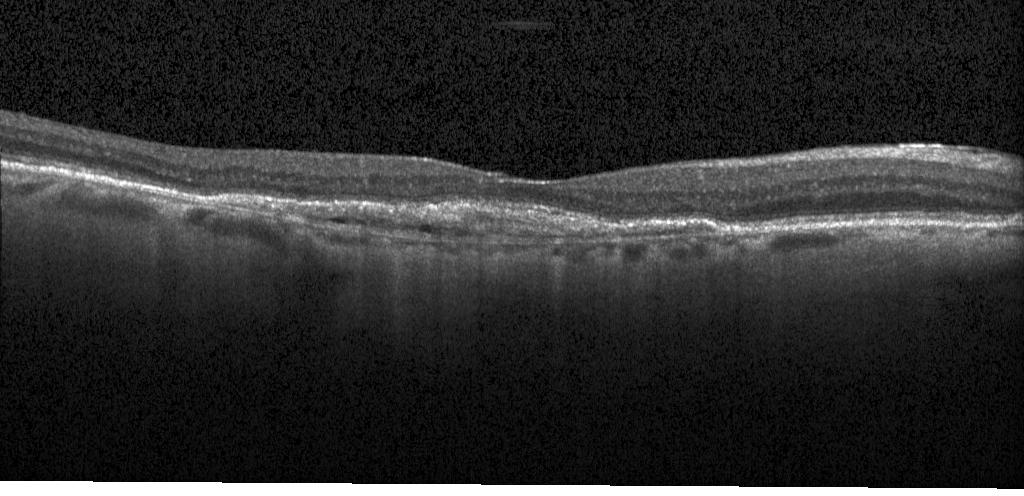 Acquired on a Heidelberg Spectralis. Optical coherence tomography scan. Through the macula — Impression: choroidal neovascularization.